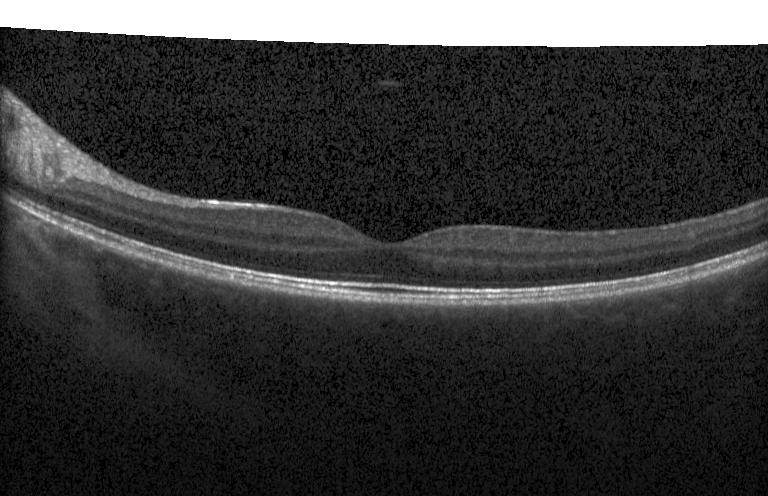

Dx: no choroidal neovascularization, diabetic macular edema, or drusen.